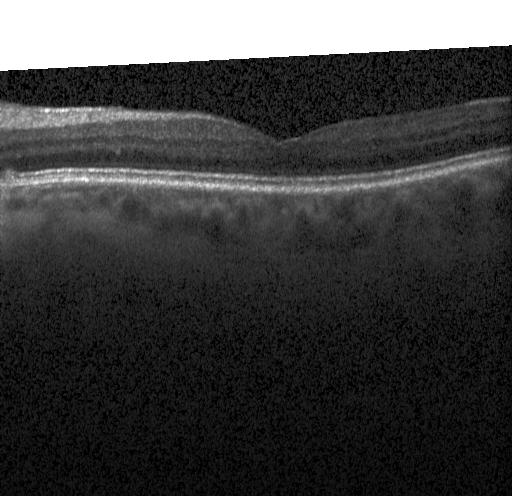
OCT B-scan
This B-scan demonstrates neither choroidal neovascularization, diabetic macular edema, nor drusen.